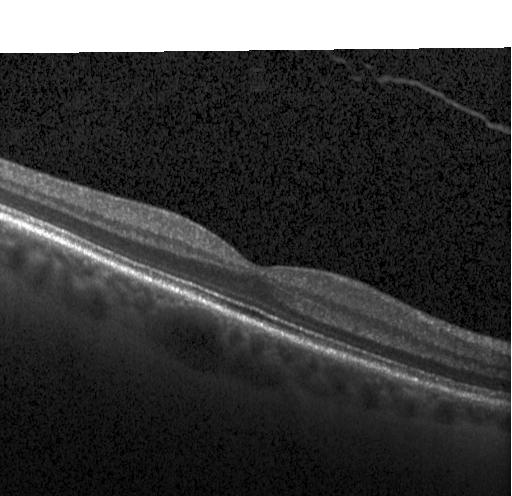 Through the macula, retinal OCT cross-section
Macular OCT: no choroidal neovascularization, diabetic macular edema, or drusen.